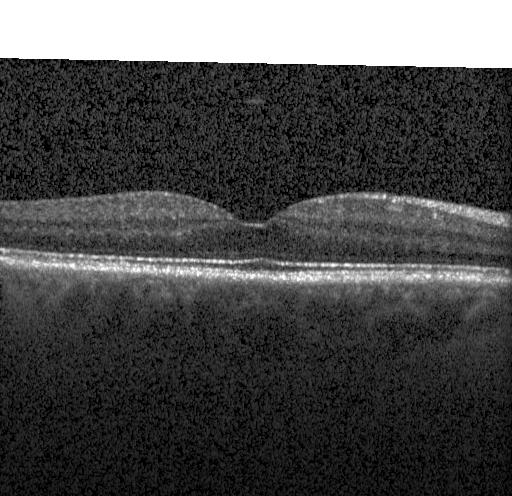
This B-scan demonstrates no choroidal neovascularization, no diabetic macular edema, and no drusen.